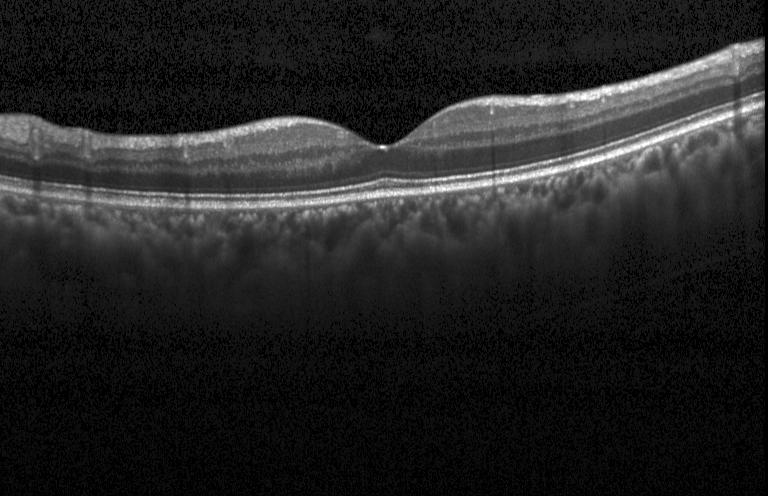 OCT B-scan — Impression: neither choroidal neovascularization, diabetic macular edema, nor drusen.